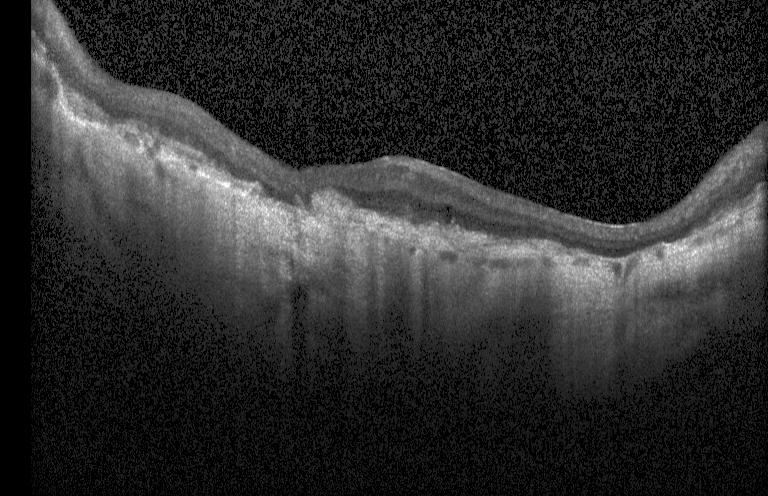 Retinal OCT B-scan, macular scan, SD-OCT
Macular OCT: choroidal neovascularization (CNV).